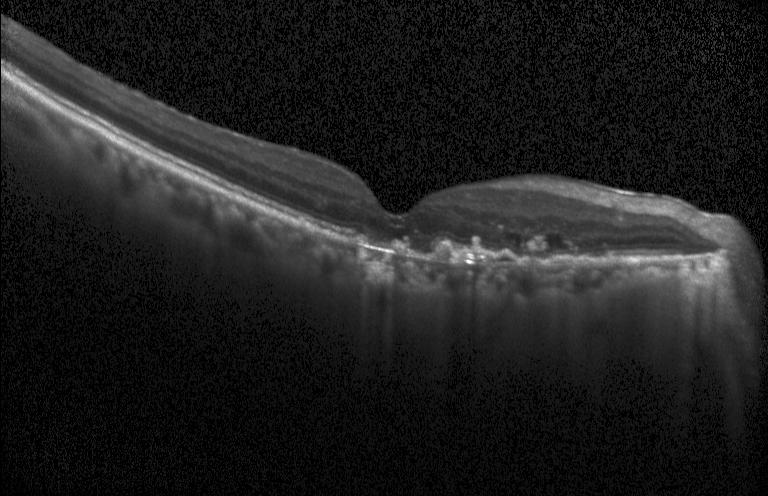

OCT B-scan, spectral-domain OCT, macular scan
Finding: choroidal neovascularization.